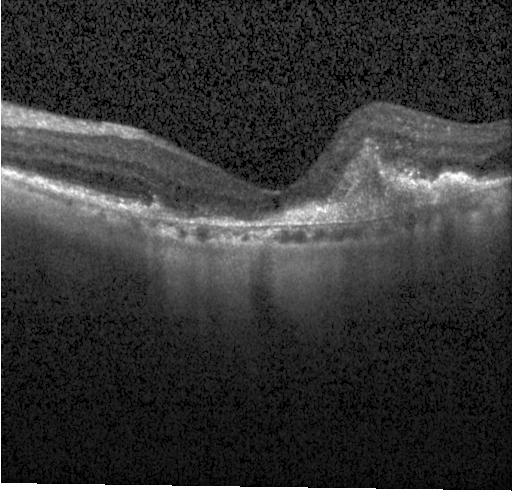

Acquired on a Heidelberg Spectralis; optical coherence tomography scan
Finding: a choroidal neovascular membrane.